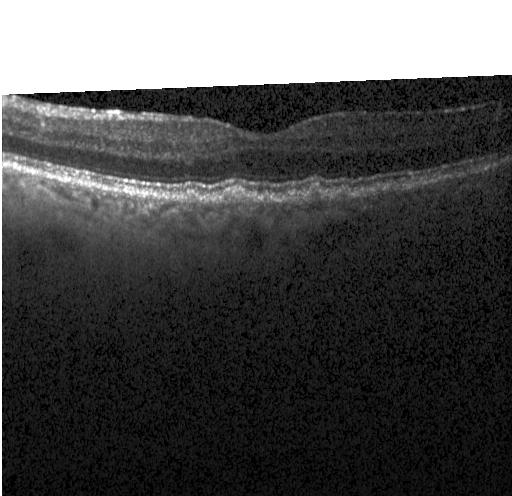
Macular OCT: sub-RPE drusenoid deposits.